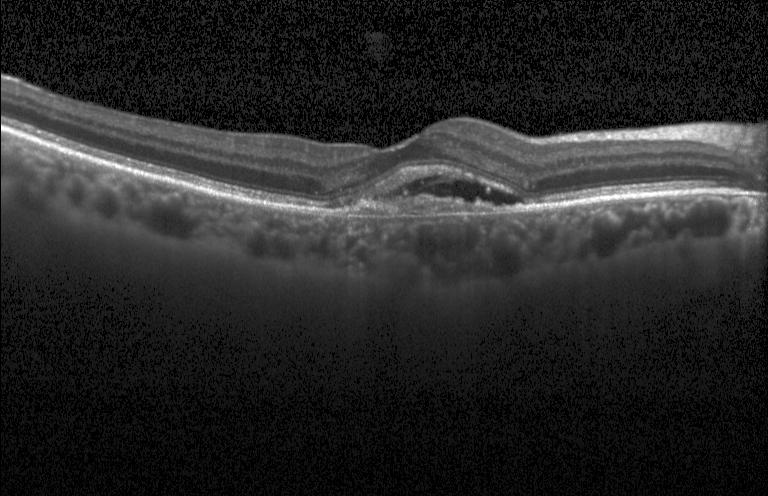
OCT finding: CNV.